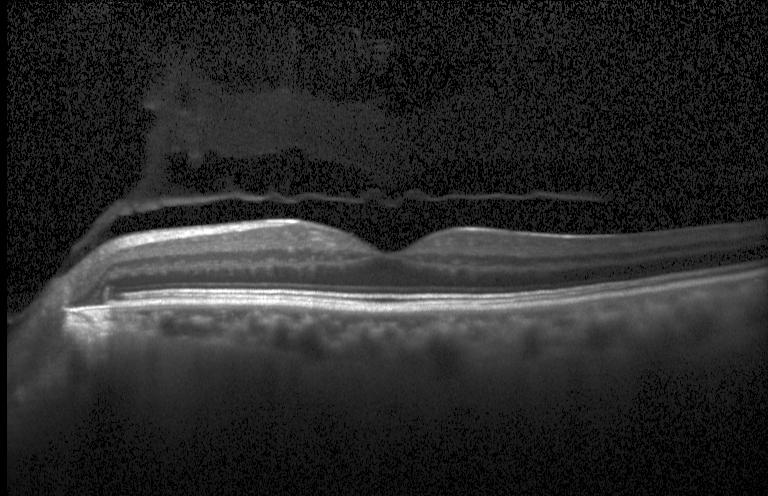 Instrument: Heidelberg Spectralis. Through the macula. Optical coherence tomography scan. SD-OCT — Dx: no choroidal neovascularization, no diabetic macular edema, and no drusen.